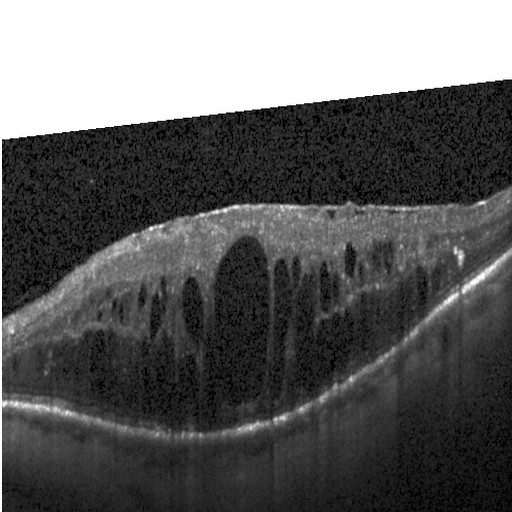 OCT scan showing DME.